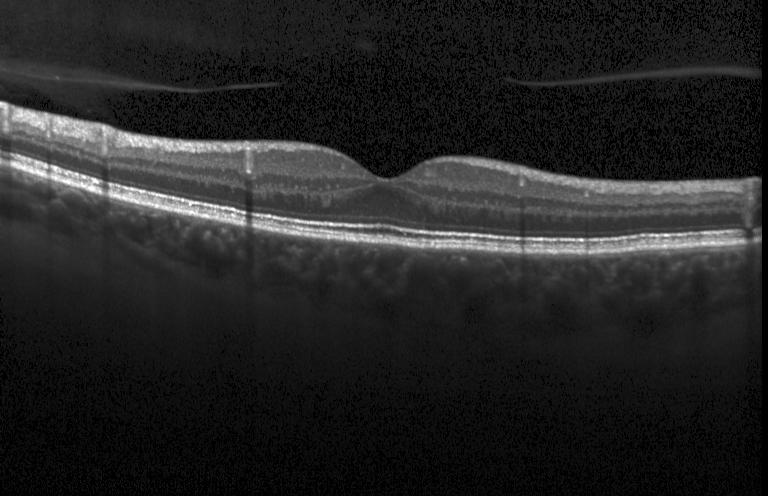 This B-scan demonstrates no evidence of choroidal neovascularization, diabetic macular edema, or drusen.